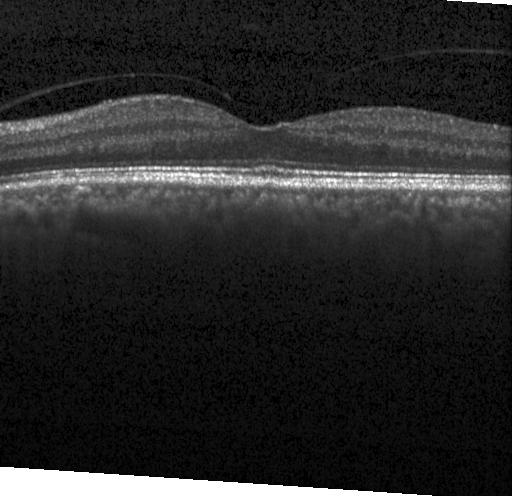
Horizontal scan through the fovea; optical coherence tomography scan
Diagnosis: neither CNV, DME, nor drusen.